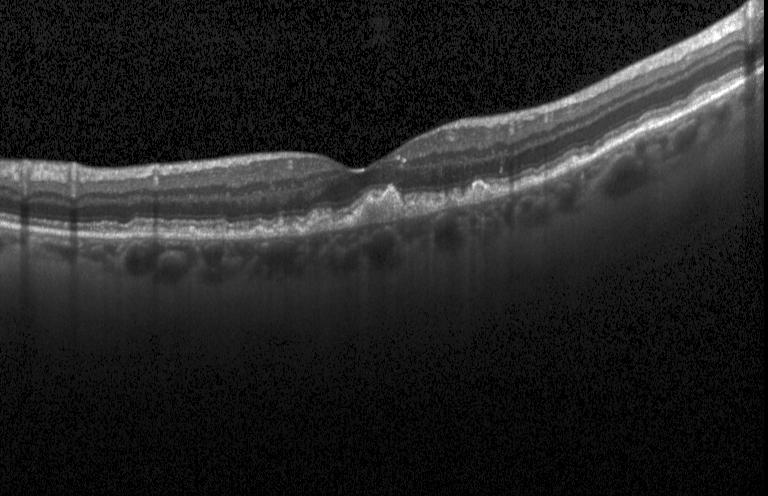
OCT B-scan. Acquired on a Heidelberg Spectralis. Impression: sub-RPE drusenoid deposits.